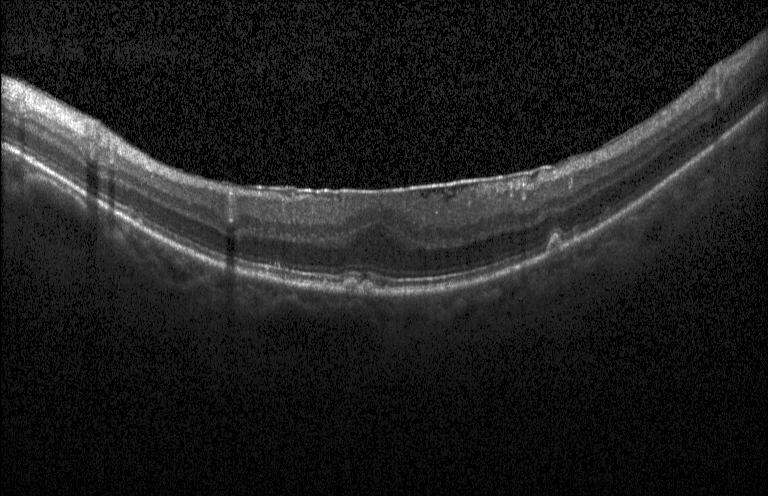
Dx: sub-RPE drusenoid deposits.